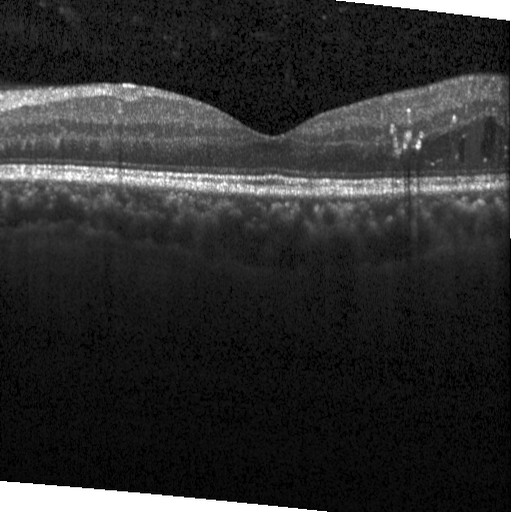
Impression: diabetic macular edema (DME).